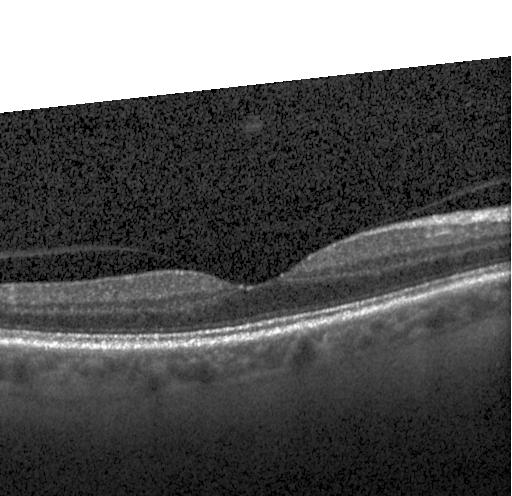 Spectral-domain OCT; optical coherence tomography scan; instrument: Heidelberg Spectralis
Assessment: no evidence of choroidal neovascularization, diabetic macular edema, or drusen.